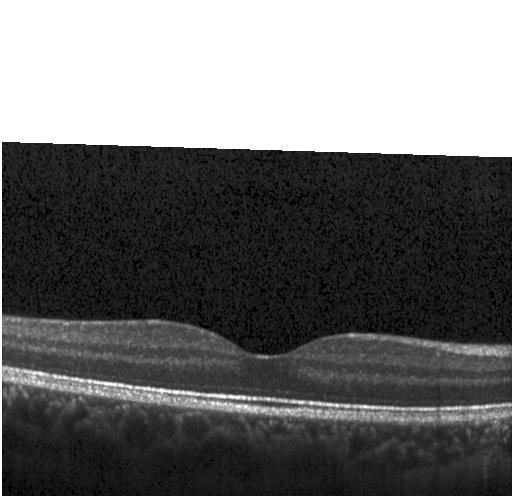 Acquired on a Heidelberg Spectralis; retinal OCT B-scan. Diagnosis: no CNV, DME, or drusen.